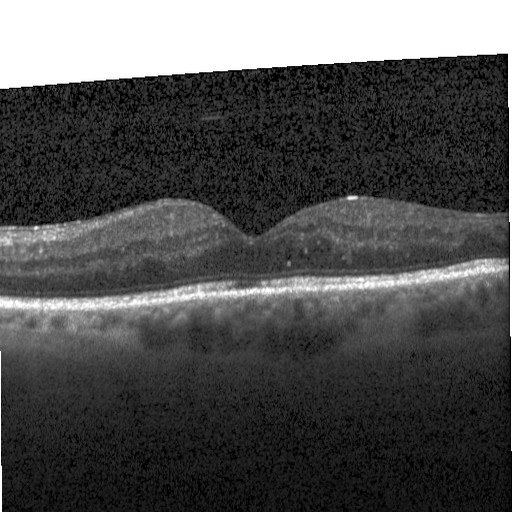 Diagnosis: DME.